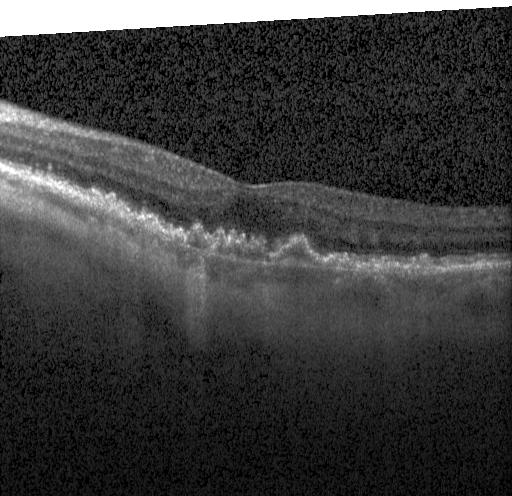

Optical coherence tomography scan
Finding: CNV.